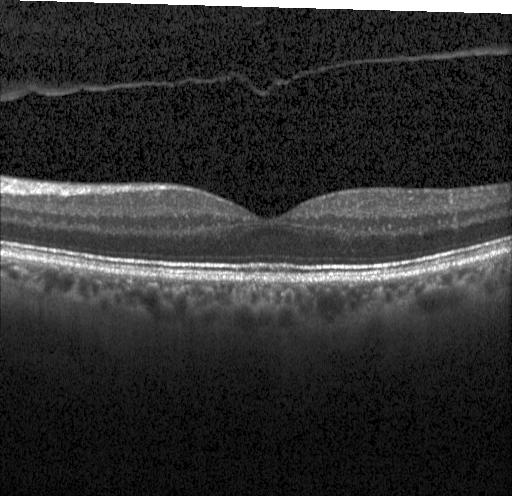 Impression: neither choroidal neovascularization, diabetic macular edema, nor drusen.